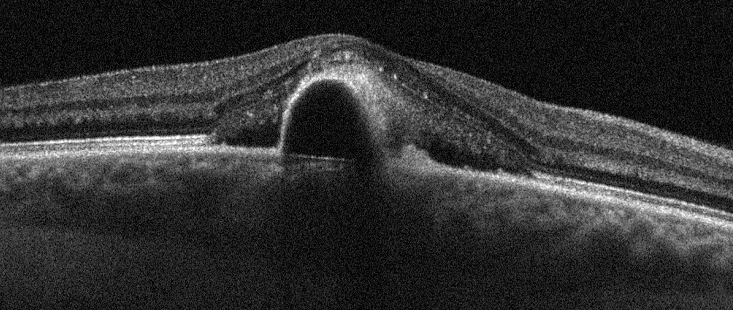 Optical coherence tomography B-scan.
Assessment: age-related macular degeneration.